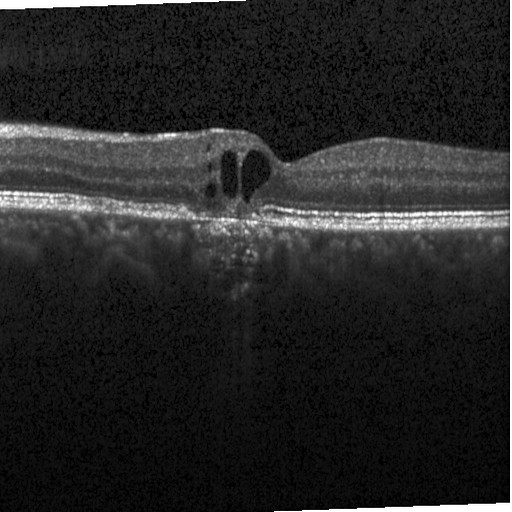 OCT line scan · acquired on a Heidelberg Spectralis · spectral-domain optical coherence tomography.
Assessment: diabetic macular edema.